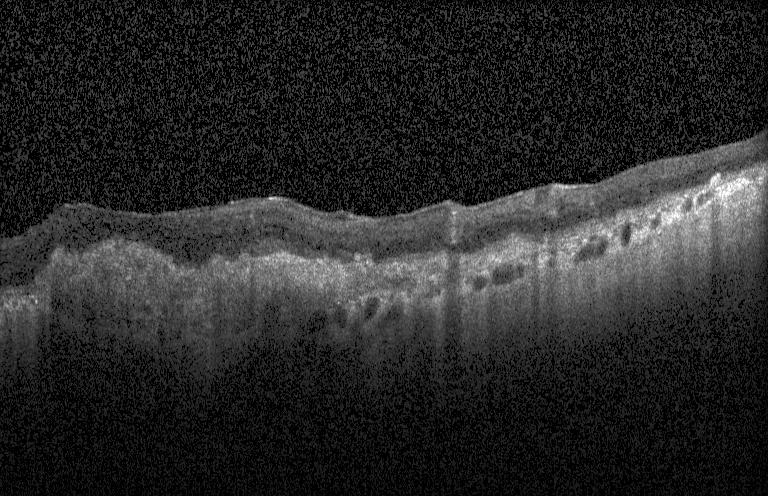
OCT finding: a choroidal neovascular membrane.